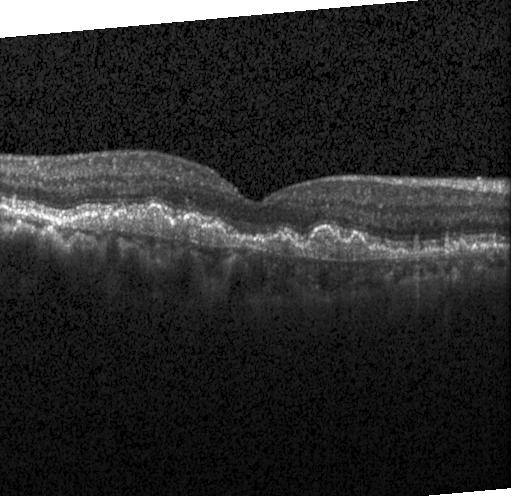
OCT scan showing choroidal neovascularization.